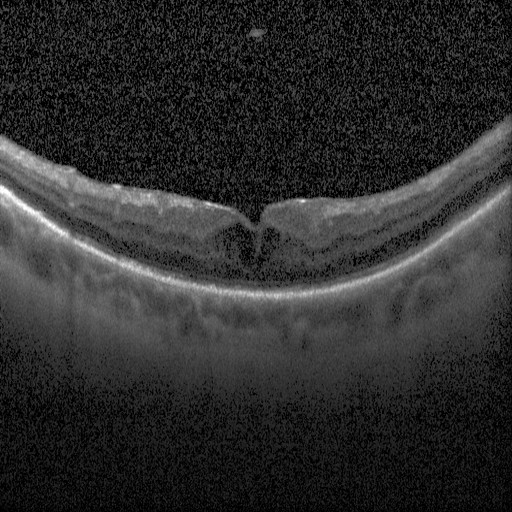

Through the macula; optical coherence tomography scan; SD-OCT; Heidelberg Spectralis. Finding: DME.